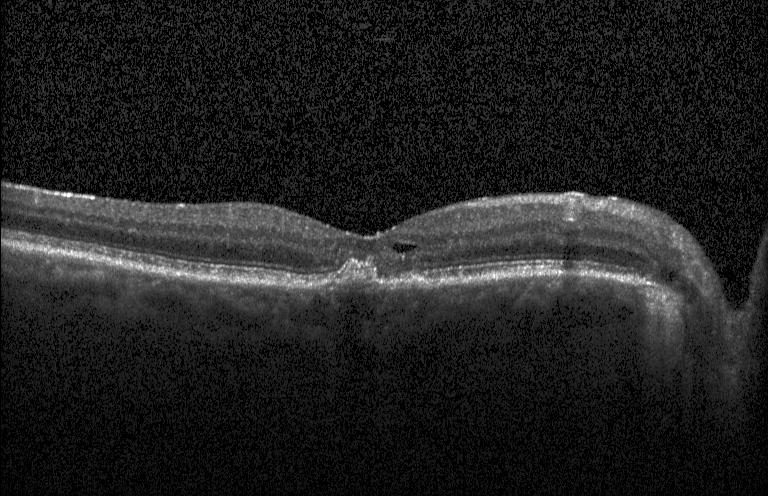

Spectral-domain optical coherence tomography · retinal OCT B-scan. Finding: a choroidal neovascular membrane.